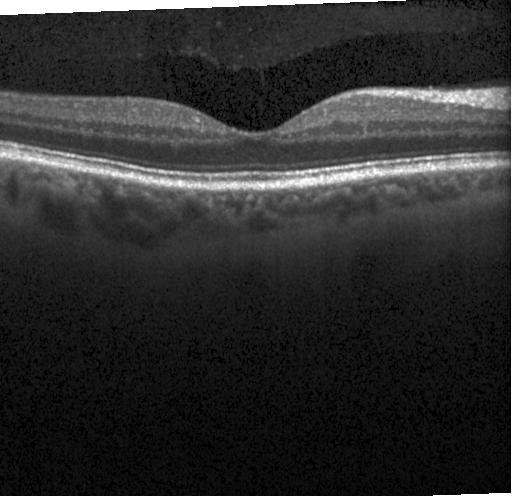 SD-OCT, optical coherence tomography B-scan — Impression: no choroidal neovascularization, no diabetic macular edema, and no drusen.